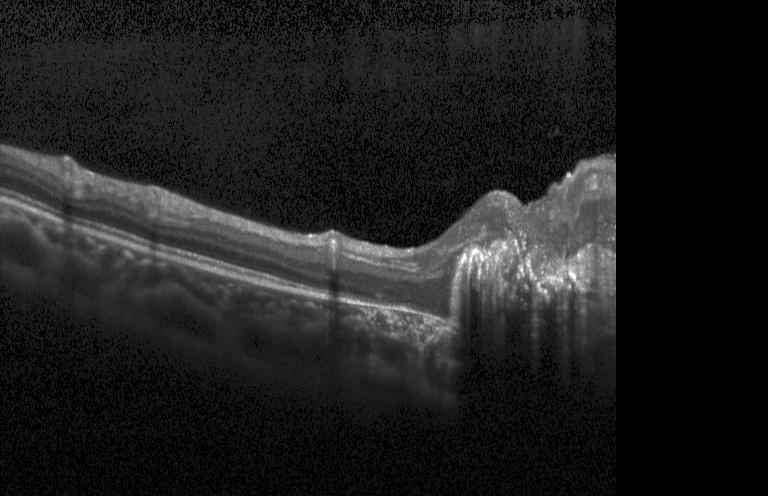

Through the macula; acquired on a Heidelberg Spectralis; optical coherence tomography scan — Choroidal neovascularization (CNV).